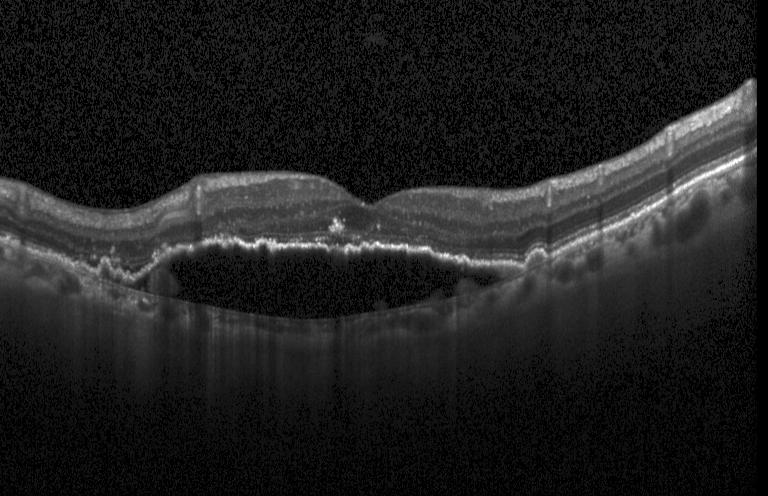
Optical coherence tomography B-scan · spectral-domain optical coherence tomography — OCT finding: a choroidal neovascular membrane.